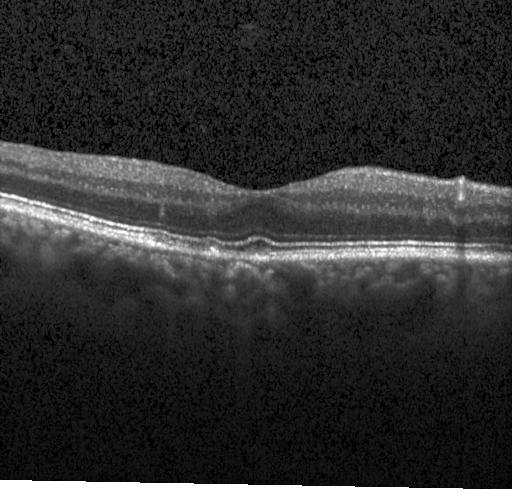
Acquired on a Heidelberg Spectralis, retinal OCT B-scan
Diagnosis: drusen.